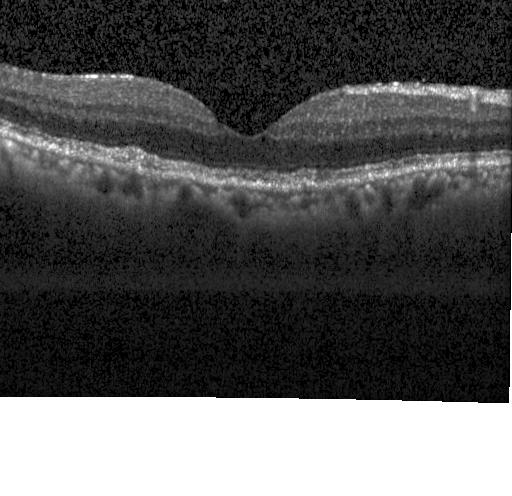 Through the macula. Spectral-domain optical coherence tomography. Acquired on a Heidelberg Spectralis. OCT B-scan
Diagnosis: multiple drusen.